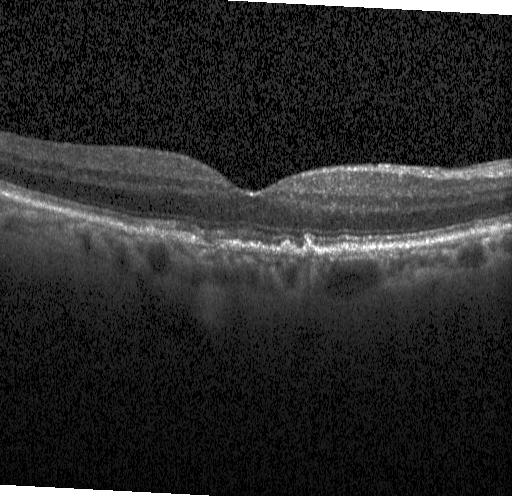

Diagnosis: drusen.